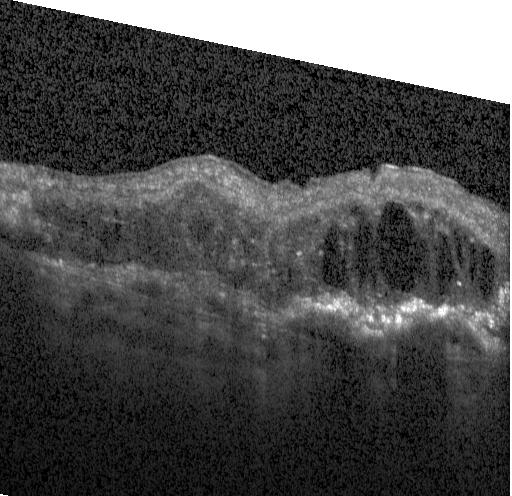

Optical coherence tomography scan; fovea-centered.
OCT finding: CNV.